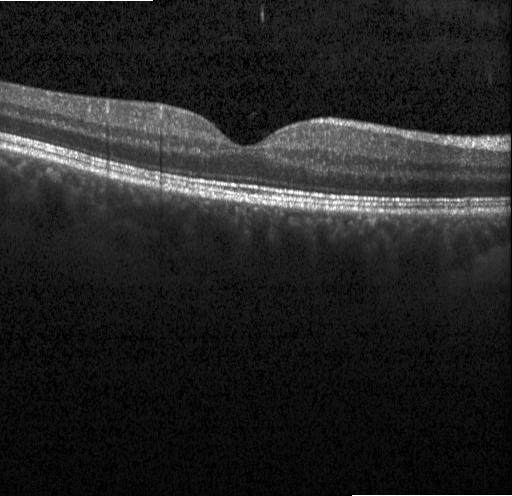 OCT finding: no CNV, DME, or drusen.